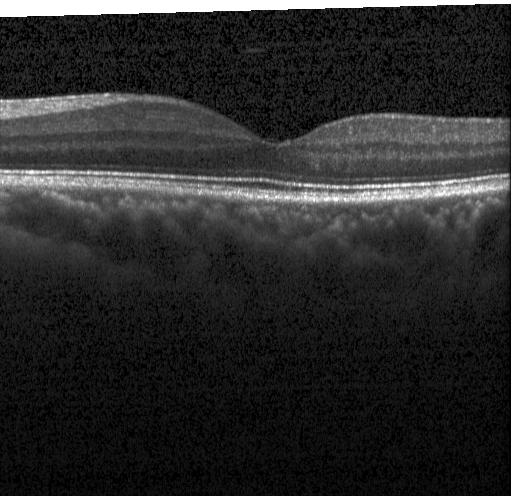 Centered on the fovea; acquired on a Heidelberg Spectralis; optical coherence tomography scan; spectral-domain optical coherence tomography. Finding: no choroidal neovascularization, diabetic macular edema, or drusen.